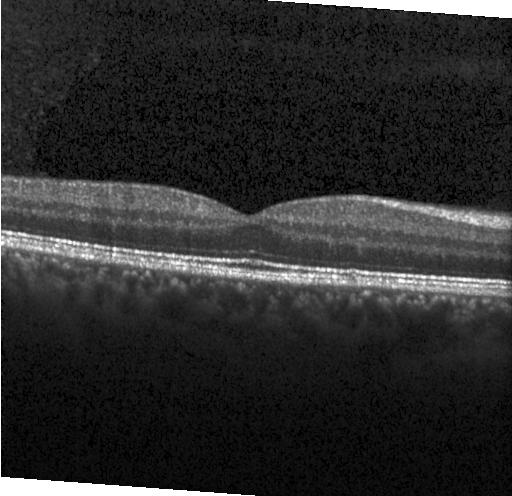 Finding: no CNV, no DME, and no drusen.